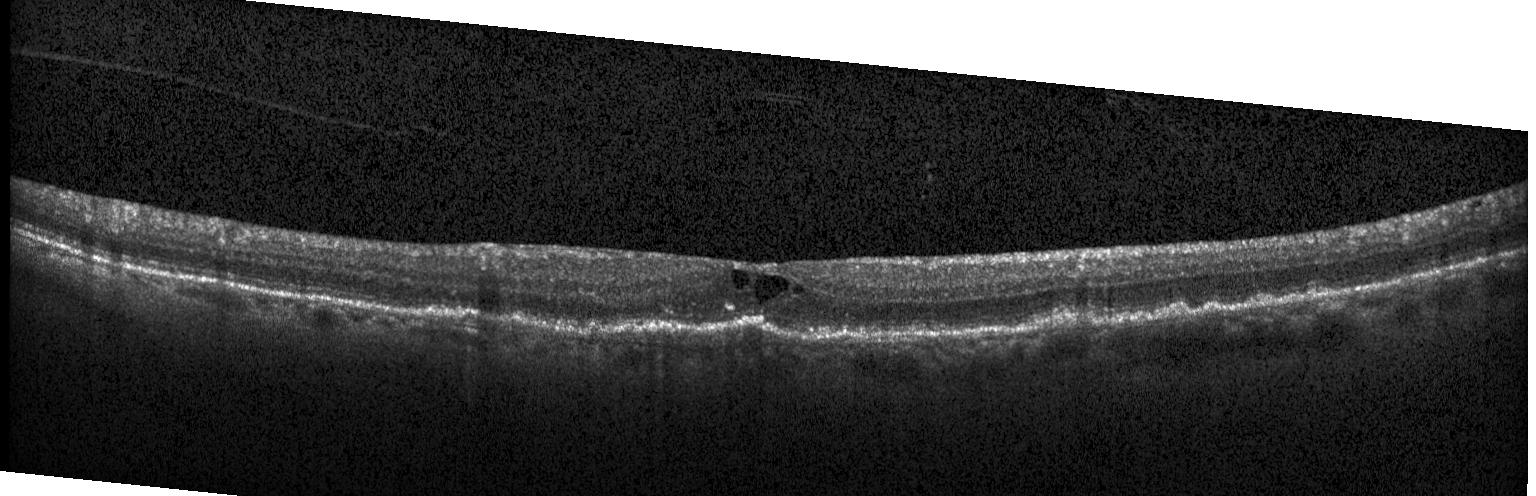 Optical coherence tomography scan. Finding: a choroidal neovascular membrane.